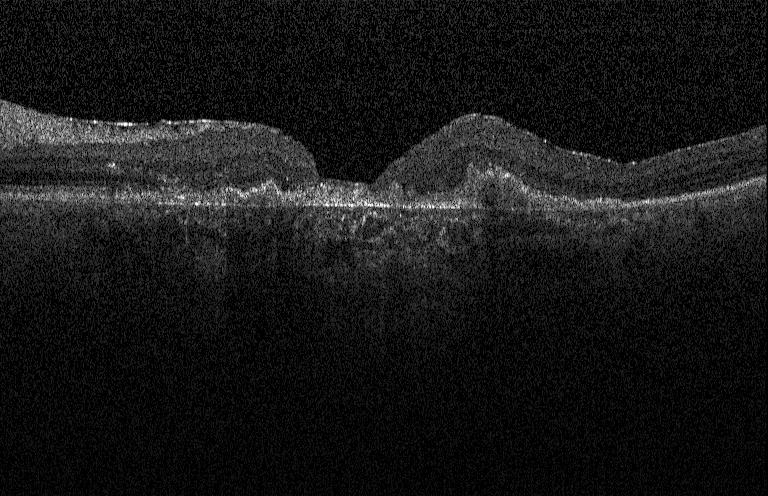 Spectral-domain OCT B-scan: choroidal neovascularization.